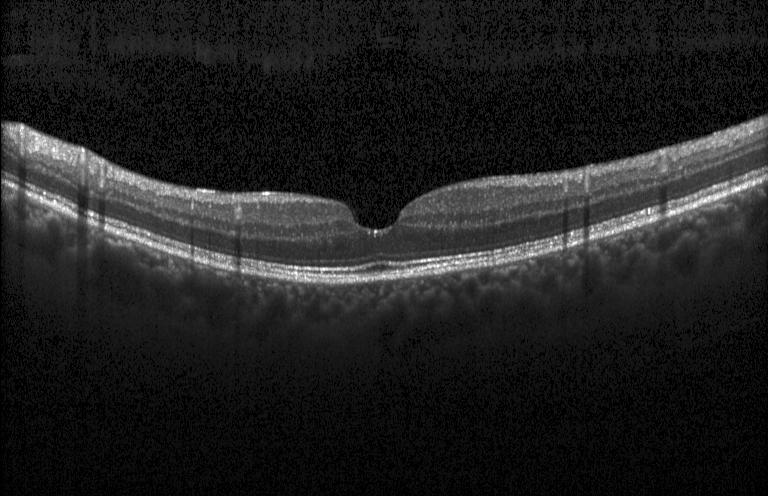

Horizontal scan through the fovea · optical coherence tomography scan · spectral-domain OCT · Heidelberg Spectralis OCT system.
Impression: no evidence of choroidal neovascularization, diabetic macular edema, or drusen.